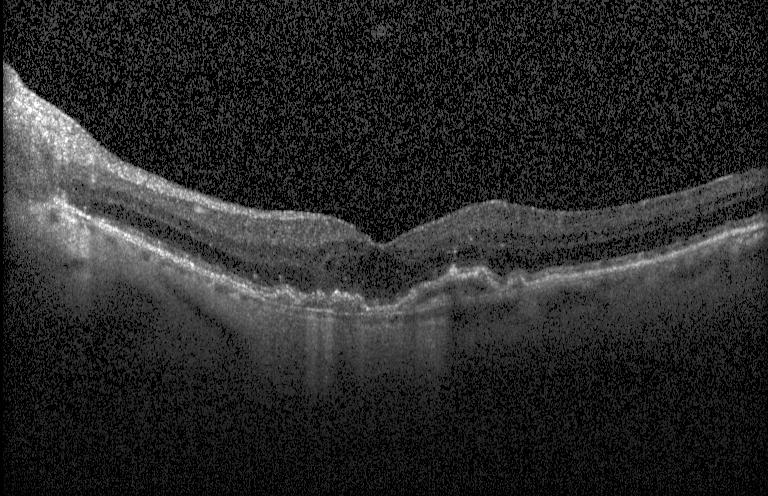 A choroidal neovascular membrane.